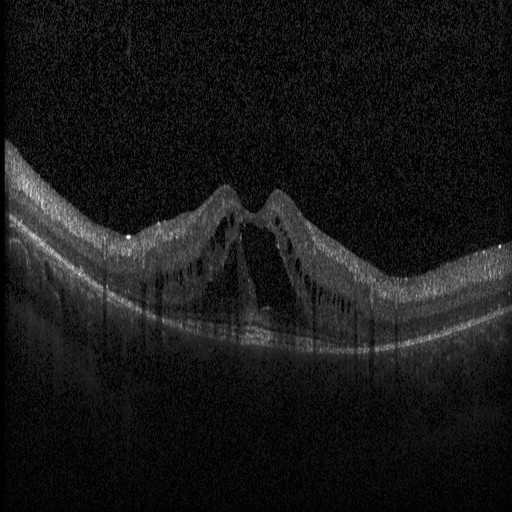
Instrument: Heidelberg Spectralis. Centered on the fovea. SD-OCT. OCT line scan
The scan shows DME.